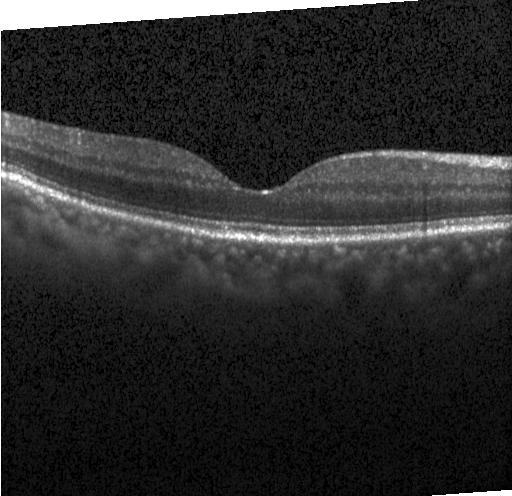 Diagnosis: no choroidal neovascularization, no diabetic macular edema, and no drusen.